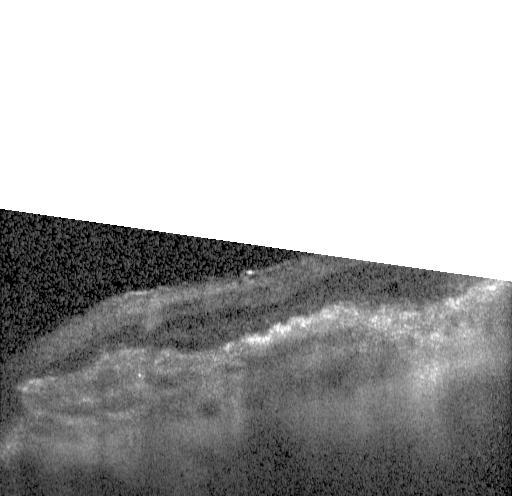 Optical coherence tomography B-scan. Horizontal scan through the fovea.
Diagnosis: a choroidal neovascular membrane.